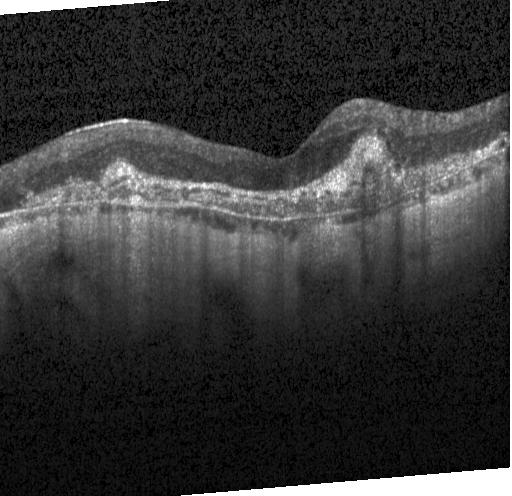
Optical coherence tomography B-scan; through the macula.
Finding: a choroidal neovascular membrane.